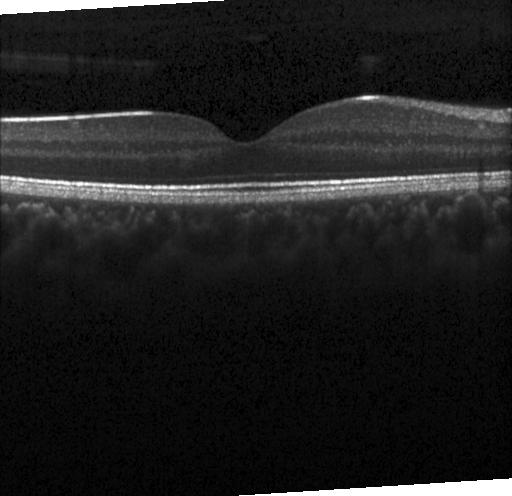 OCT finding: no CNV, no DME, and no drusen.